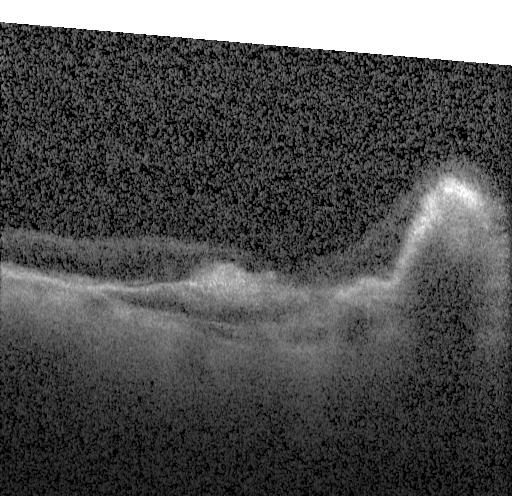 Macular scan, optical coherence tomography scan.
Macular OCT: a choroidal neovascular membrane.